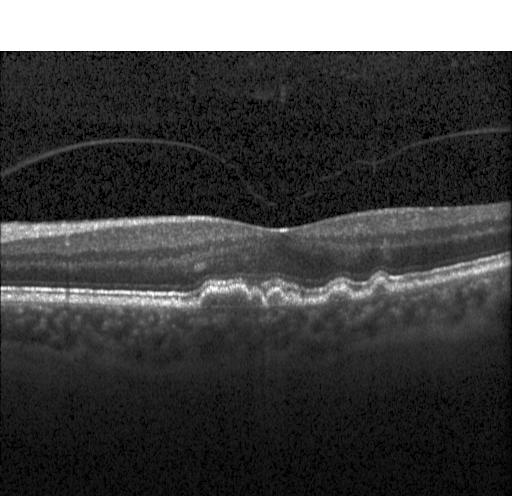

OCT finding: sub-RPE drusenoid deposits.